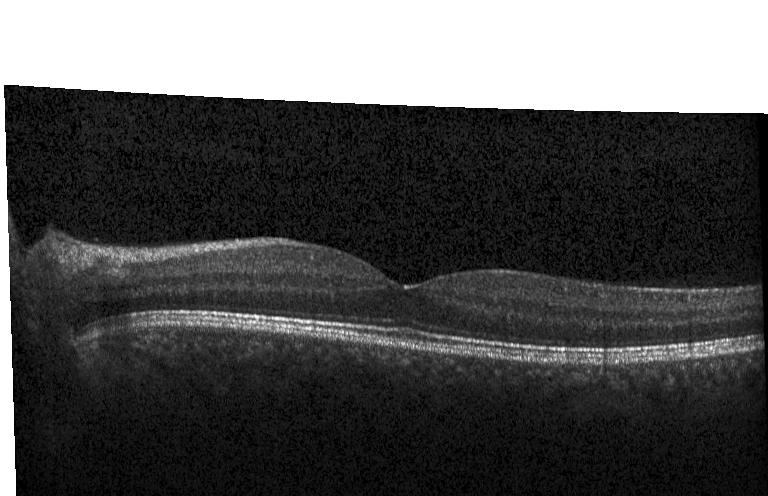 Fovea-centered; optical coherence tomography scan; spectral-domain OCT.
This B-scan demonstrates no CNV, no DME, and no drusen.